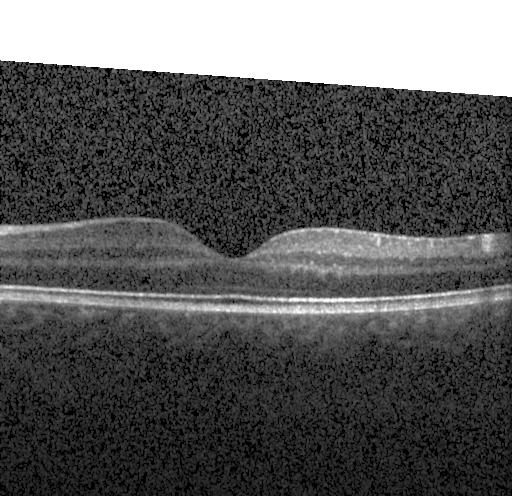 SD-OCT. Optical coherence tomography scan.
Finding: no CNV, DME, or drusen.